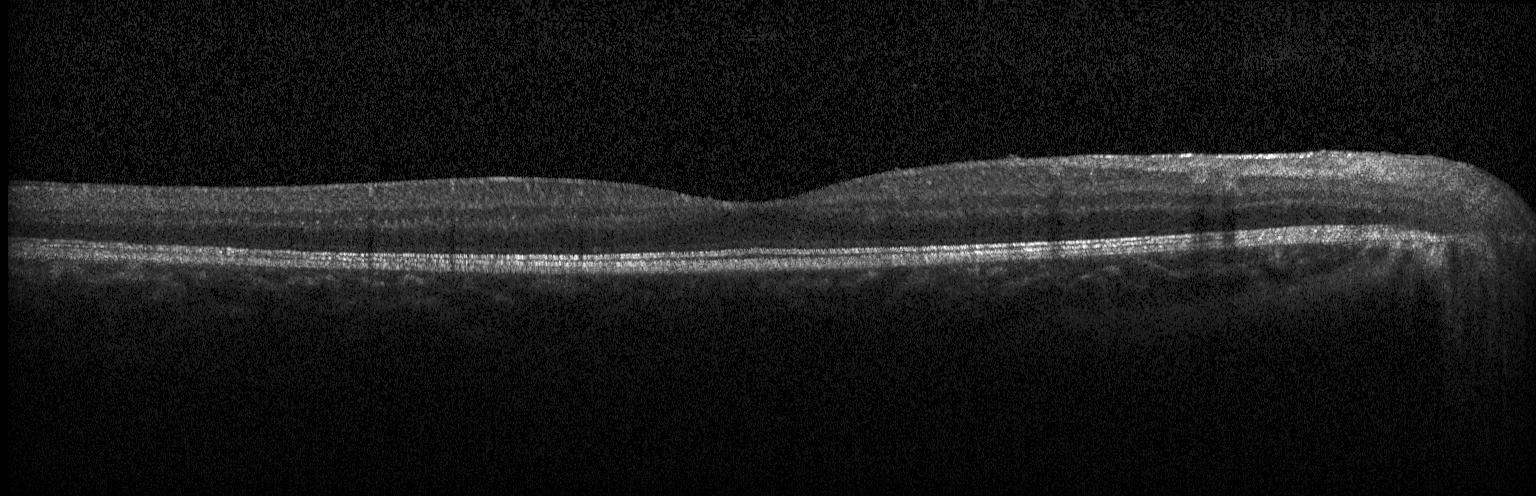 OCT B-scan showing no choroidal neovascularization, no diabetic macular edema, and no drusen.